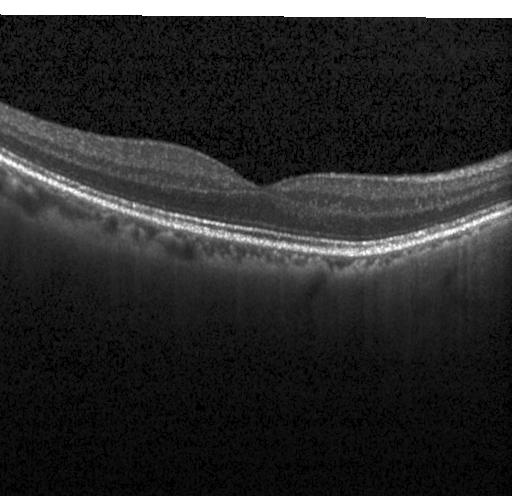 Impression: neither CNV, DME, nor drusen.